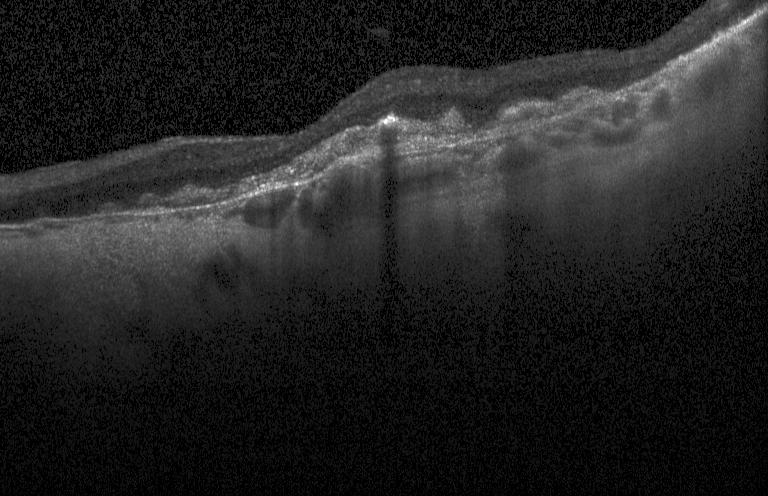
Spectral-domain optical coherence tomography · retinal OCT B-scan · instrument: Heidelberg Spectralis.
A choroidal neovascular membrane.